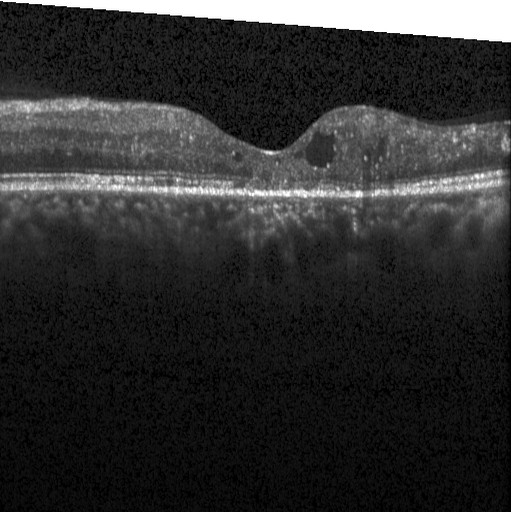 SD-OCT · OCT line scan
Finding: diabetic macular edema.